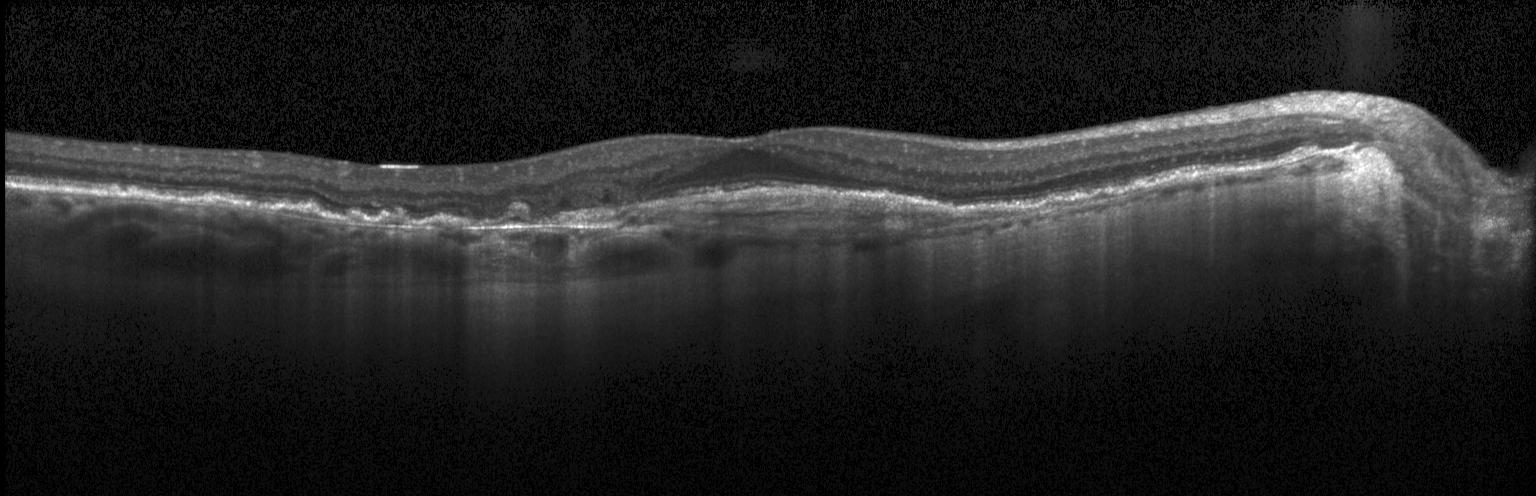

Diagnosis: choroidal neovascularization.